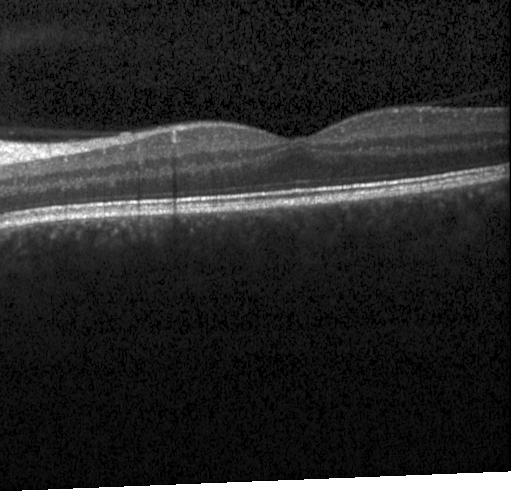 Retinal OCT cross-section · Heidelberg Spectralis OCT system · spectral-domain OCT.
Diagnosis: no evidence of CNV, DME, or drusen.